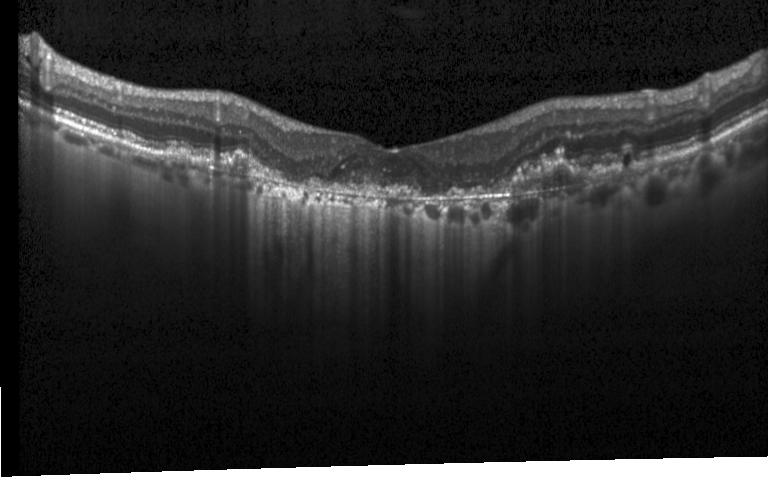
Optical coherence tomography B-scan.
Diagnosis: choroidal neovascularization (CNV).